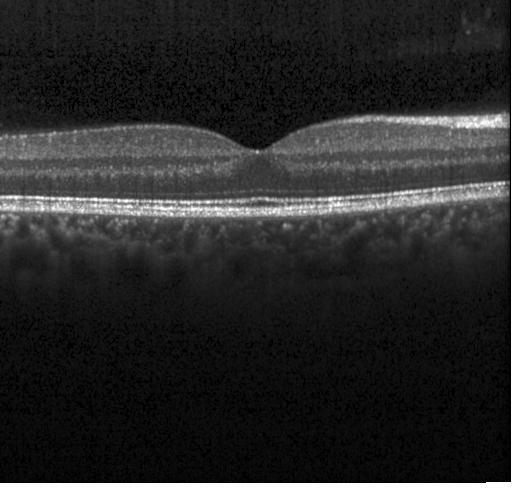

The scan shows no CNV, no DME, and no drusen.